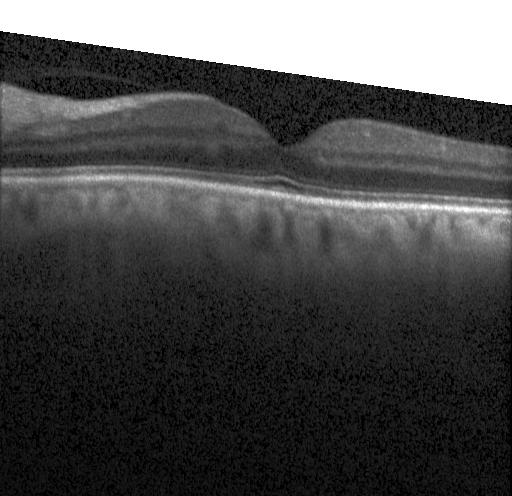 Instrument: Heidelberg Spectralis. Retinal OCT cross-section.
Diagnosis: no choroidal neovascularization, no diabetic macular edema, and no drusen.